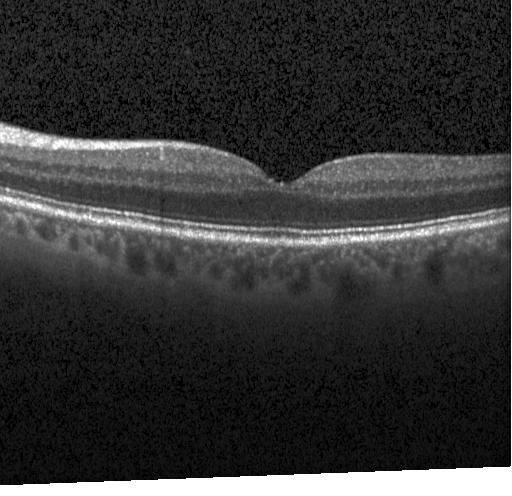
Acquired on a Heidelberg Spectralis. Optical coherence tomography B-scan. The scan shows neither choroidal neovascularization, diabetic macular edema, nor drusen.